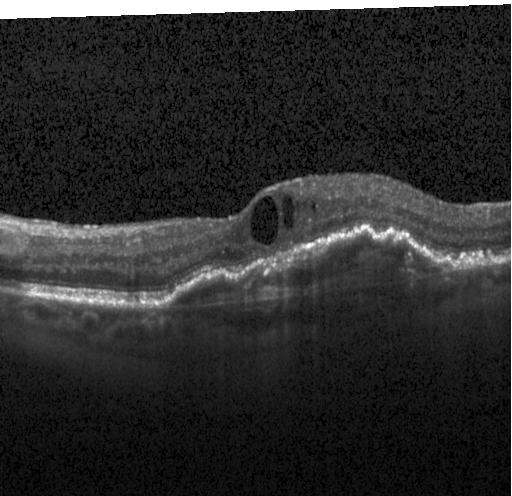
OCT scan showing choroidal neovascularization (CNV).